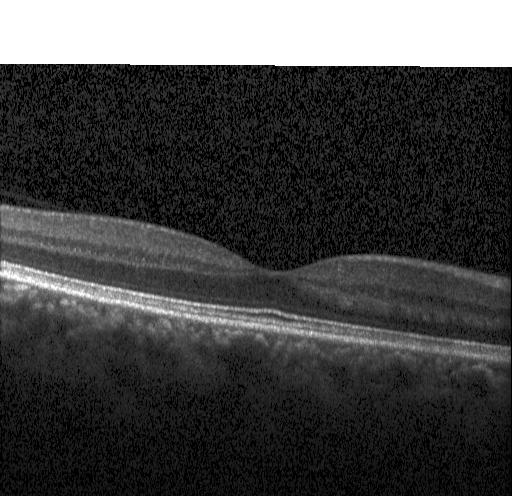
OCT line scan; macular scan
Neither choroidal neovascularization, diabetic macular edema, nor drusen.